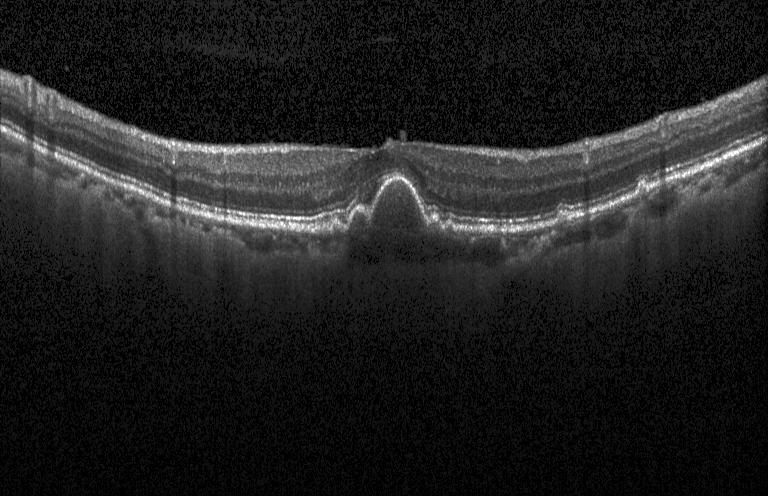 Finding: CNV.